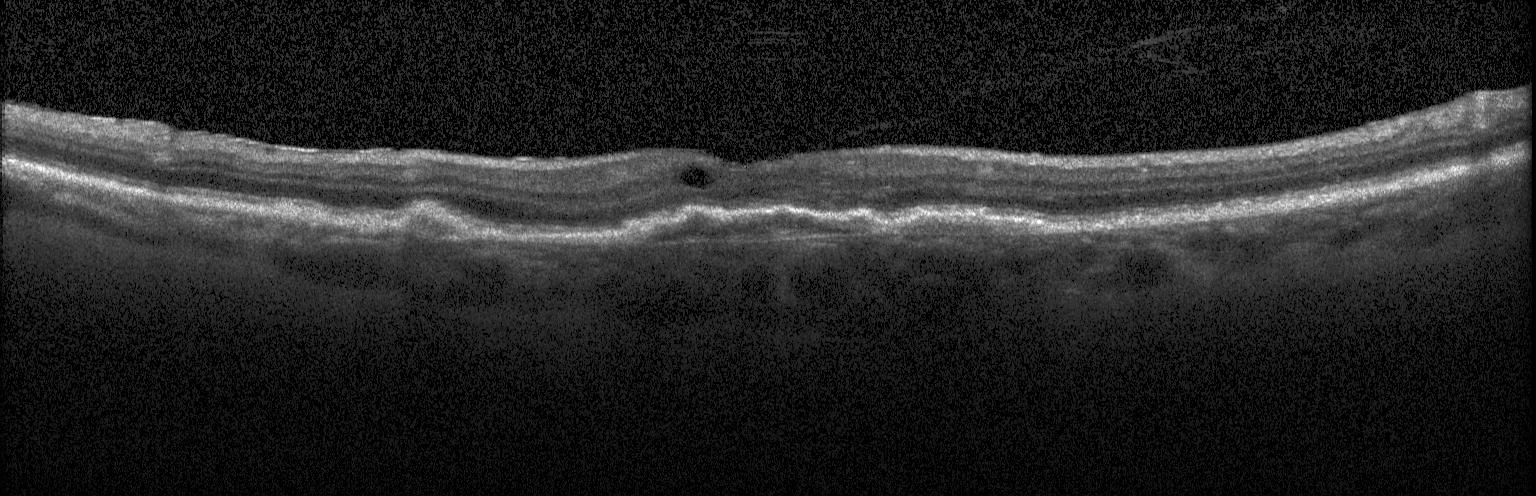
SD-OCT. Instrument: Heidelberg Spectralis. Optical coherence tomography B-scan. Horizontal scan through the fovea. Impression: a choroidal neovascular membrane.